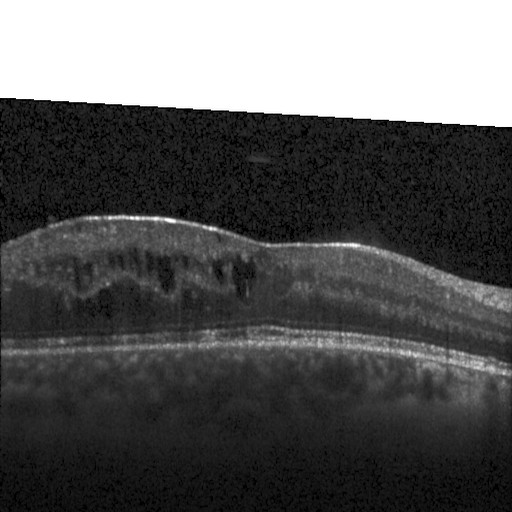
Through the macula · spectral-domain optical coherence tomography · OCT B-scan — The scan shows diabetic macular edema.